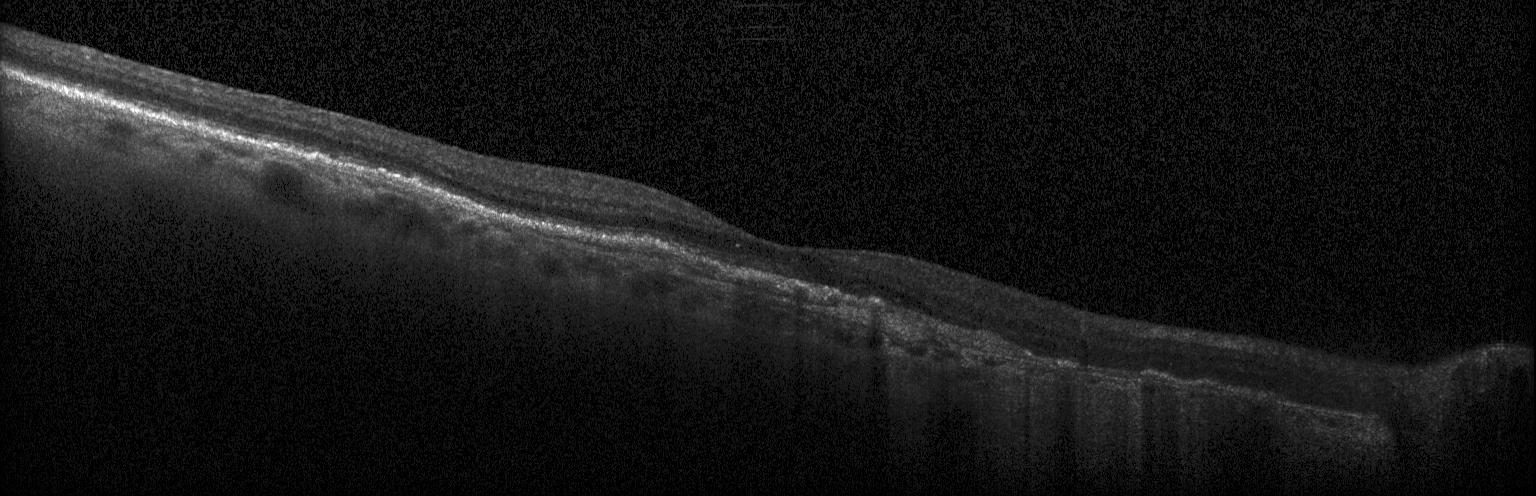 Spectral-domain OCT B-scan: a choroidal neovascular membrane.